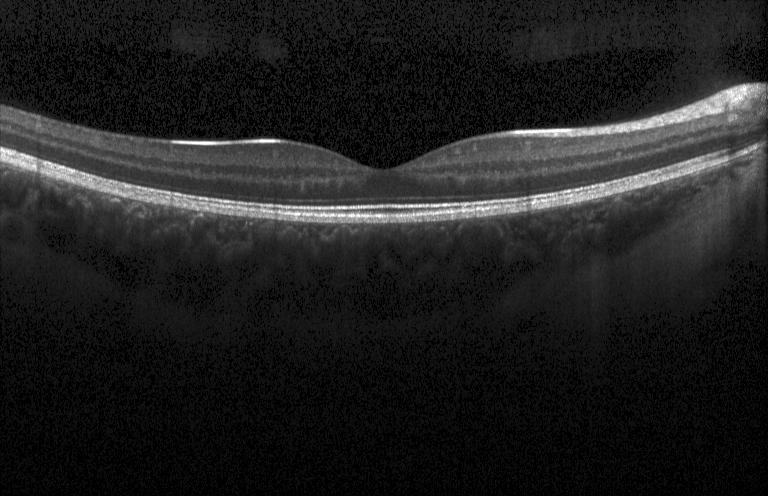
Heidelberg Spectralis; centered on the fovea; OCT B-scan; spectral-domain OCT
The scan shows no CNV, no DME, and no drusen.